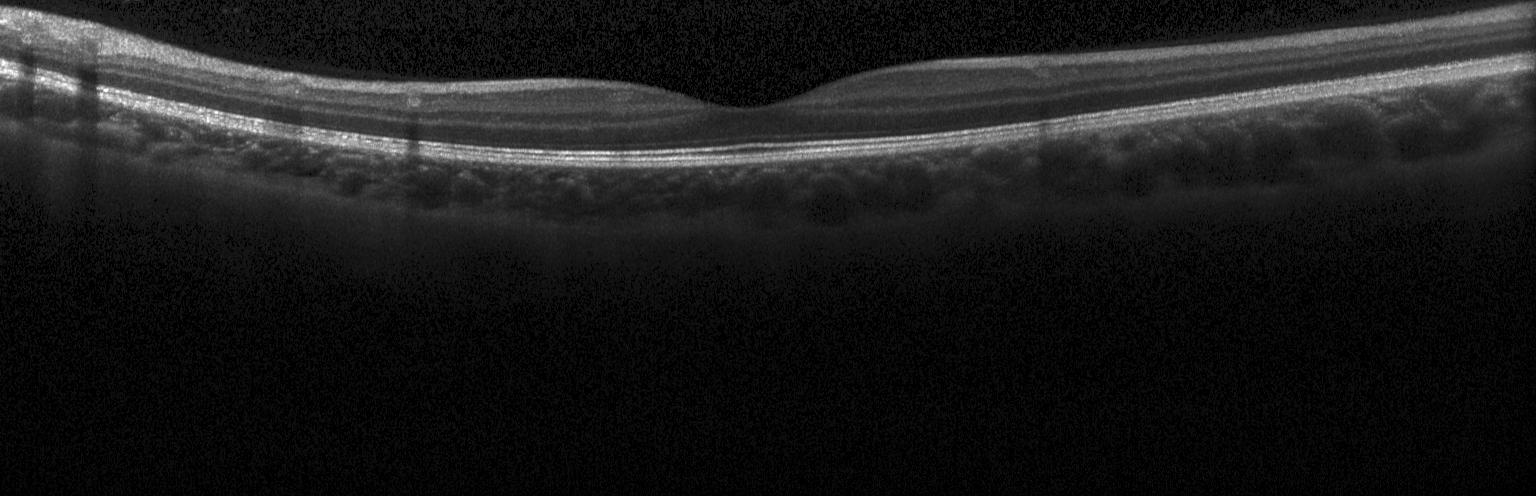 Acquired on a Heidelberg Spectralis; macular scan; optical coherence tomography B-scan
This B-scan demonstrates neither CNV, DME, nor drusen.